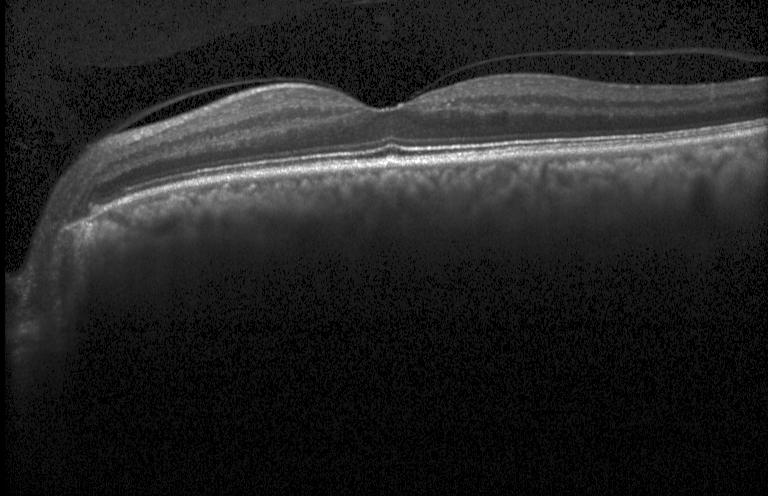

Finding: no CNV, no DME, and no drusen.